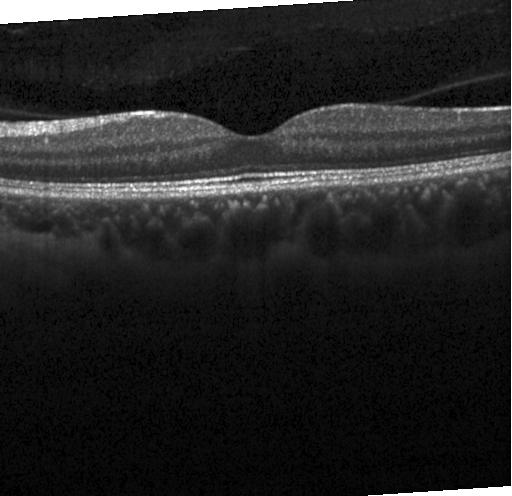
No evidence of choroidal neovascularization, diabetic macular edema, or drusen.